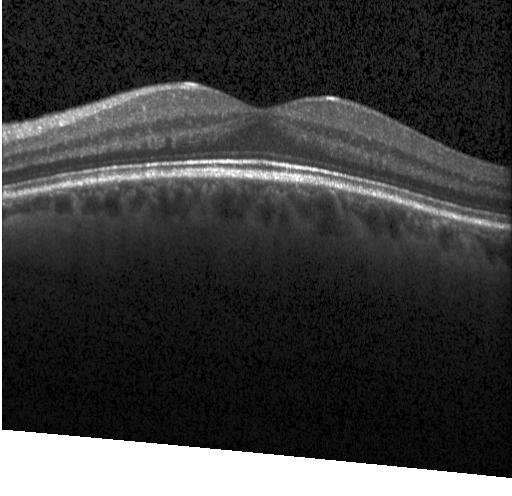 Spectral-domain OCT B-scan: no choroidal neovascularization, diabetic macular edema, or drusen.